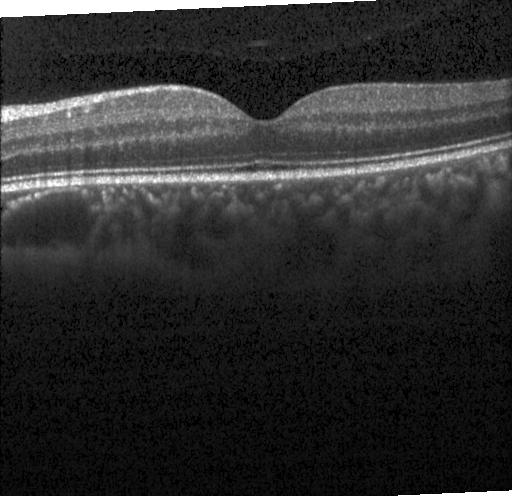

OCT B-scan.
No CNV, no DME, and no drusen.